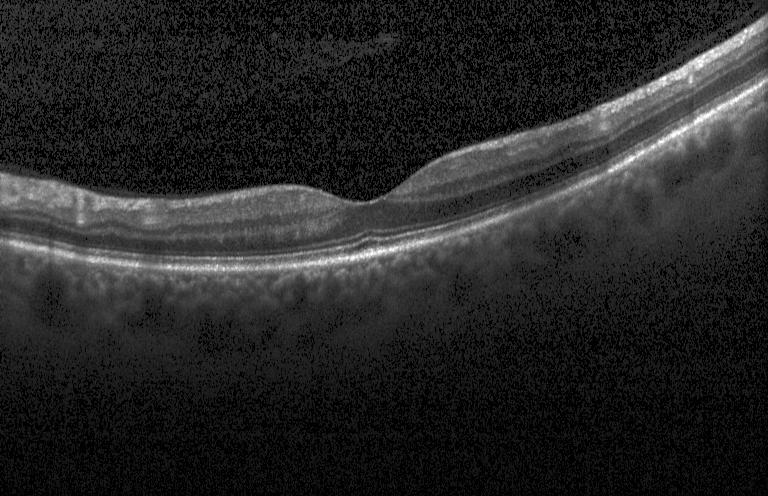
Impression: no choroidal neovascularization, diabetic macular edema, or drusen.